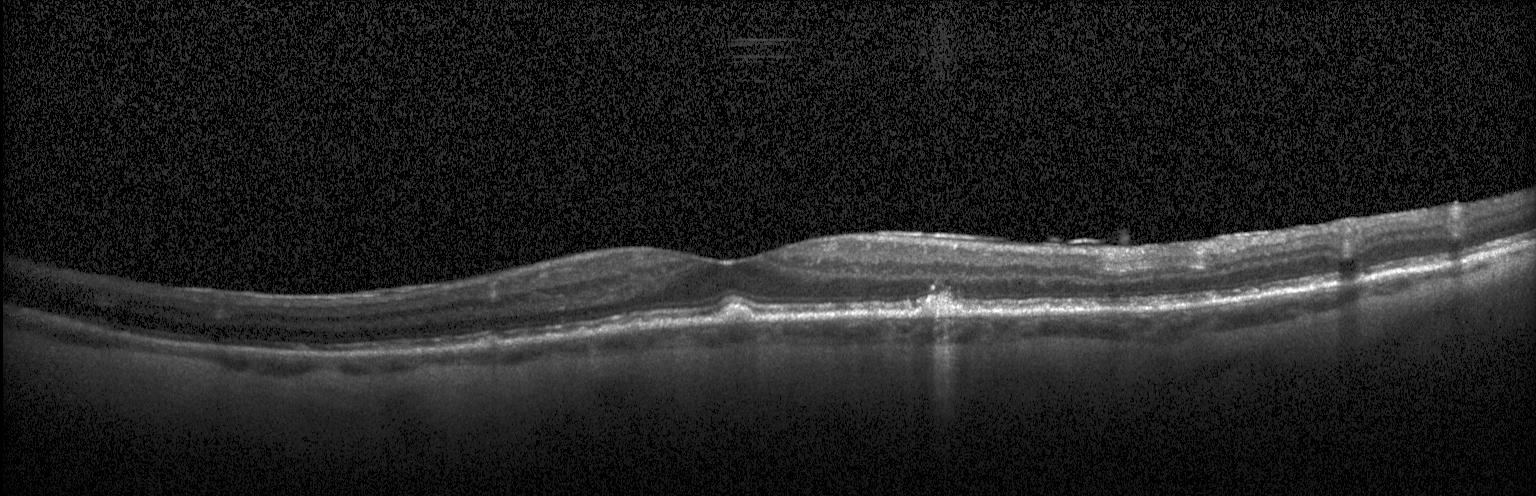
Diagnosis: drusen.